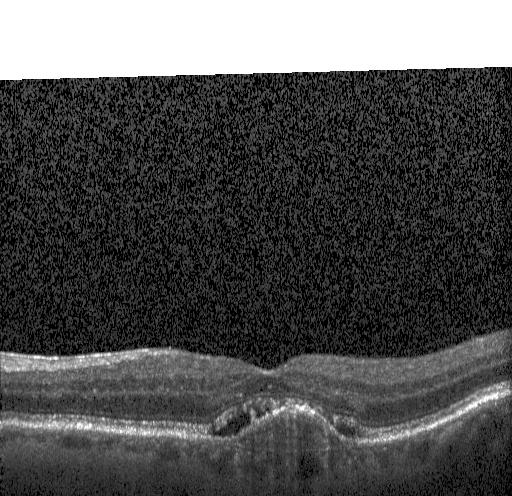
Spectral-domain optical coherence tomography. OCT B-scan — Diagnosis: a choroidal neovascular membrane.